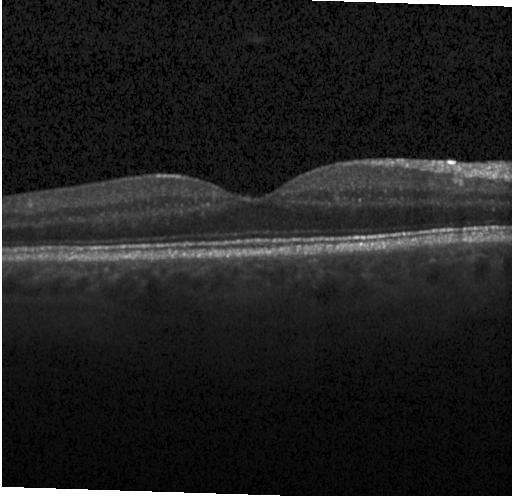 Optical coherence tomography scan — Dx: no evidence of CNV, DME, or drusen.